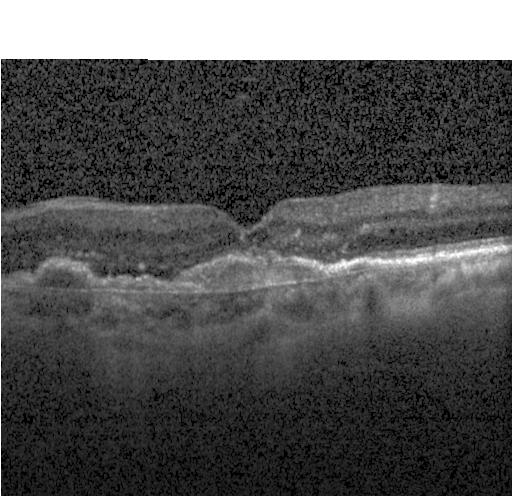

Optical coherence tomography scan.
Finding: a choroidal neovascular membrane.